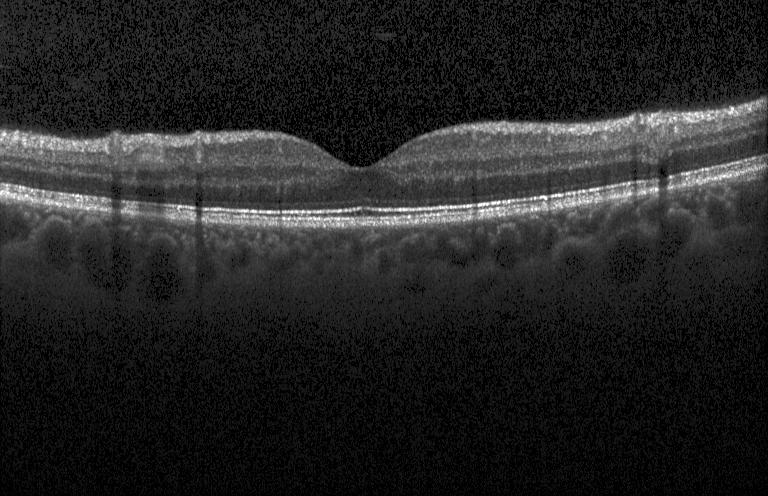 Heidelberg Spectralis OCT system; optical coherence tomography B-scan; SD-OCT; horizontal scan through the fovea.
Macular OCT: no choroidal neovascularization, no diabetic macular edema, and no drusen.